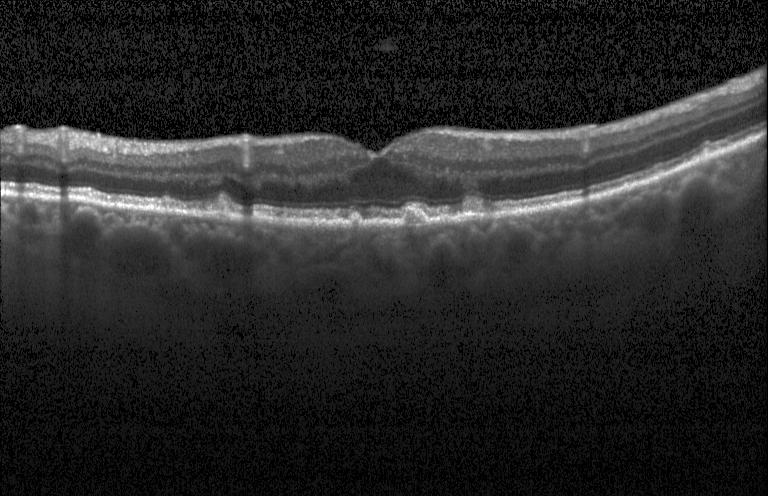
Macular OCT demonstrating sub-RPE drusenoid deposits.